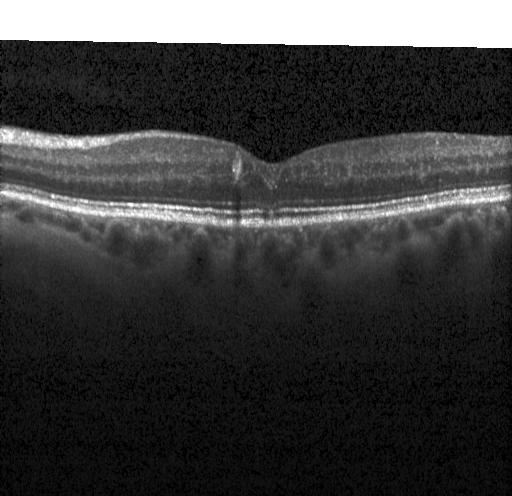 Diagnosis: no evidence of CNV, DME, or drusen.